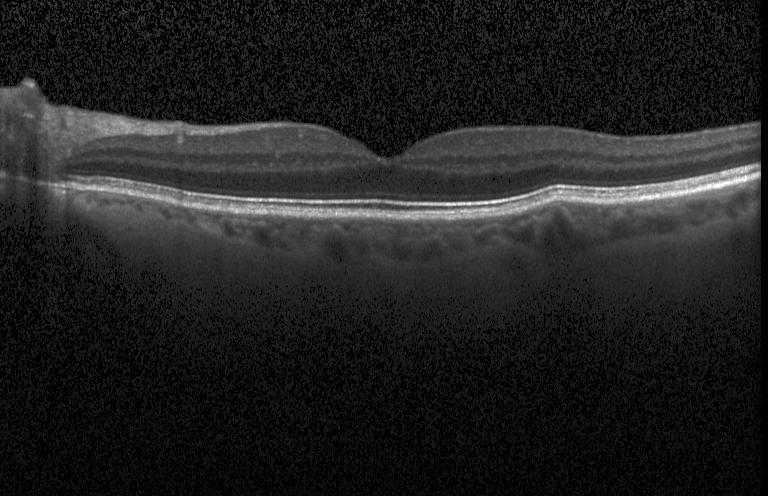
Optical coherence tomography B-scan, spectral-domain OCT, macular scan, Heidelberg Spectralis — Impression: no CNV, DME, or drusen.